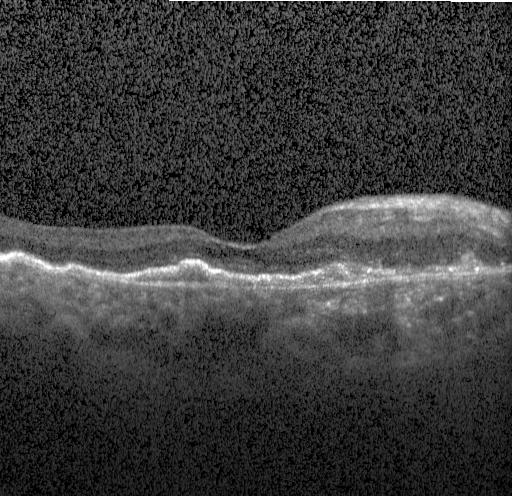
Optical coherence tomography scan, macular scan, SD-OCT, acquired on a Heidelberg Spectralis — This B-scan demonstrates CNV.